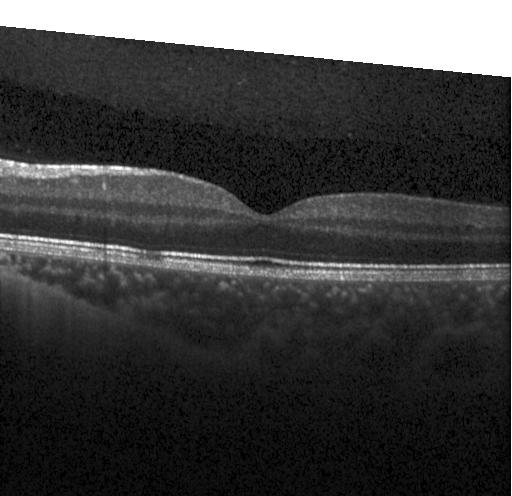
Finding: no evidence of choroidal neovascularization, diabetic macular edema, or drusen.